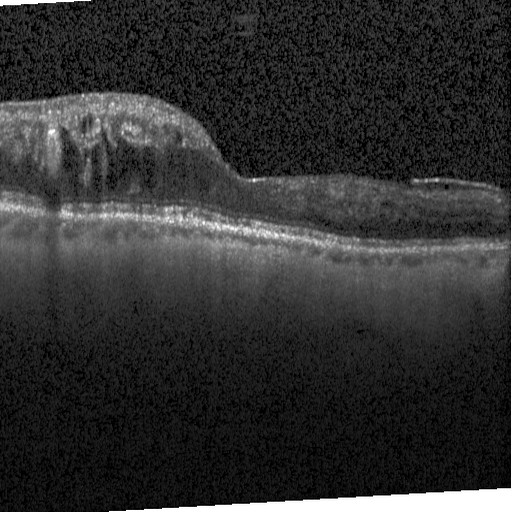

Centered on the fovea, Heidelberg Spectralis OCT system, optical coherence tomography B-scan.
This B-scan demonstrates DME.